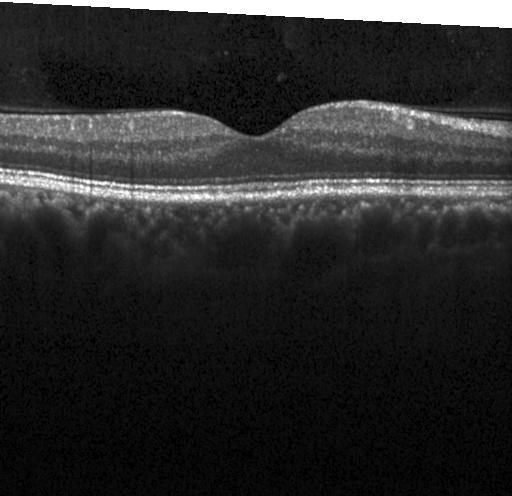
Impression: no CNV, no DME, and no drusen.